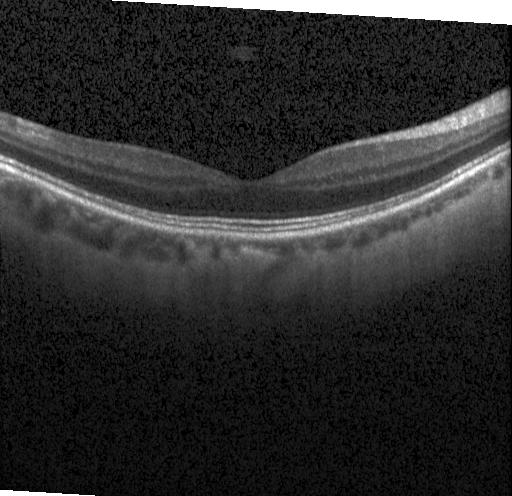

Horizontal scan through the fovea; optical coherence tomography scan
Assessment: no evidence of CNV, DME, or drusen.